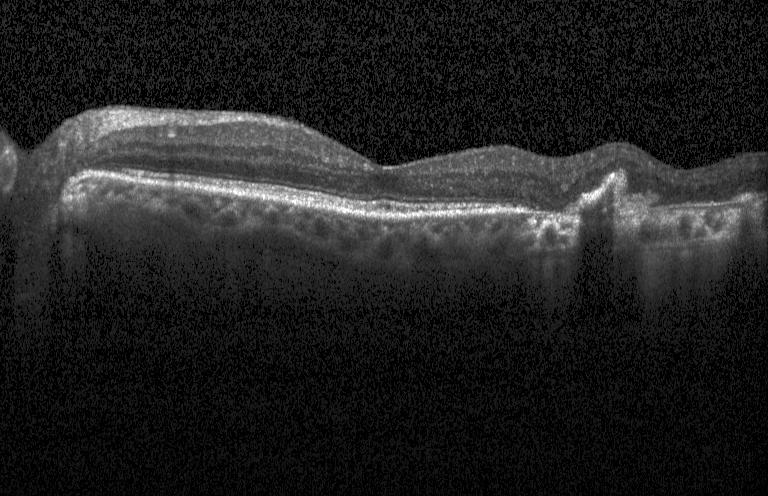
OCT line scan — The scan shows choroidal neovascularization (CNV).